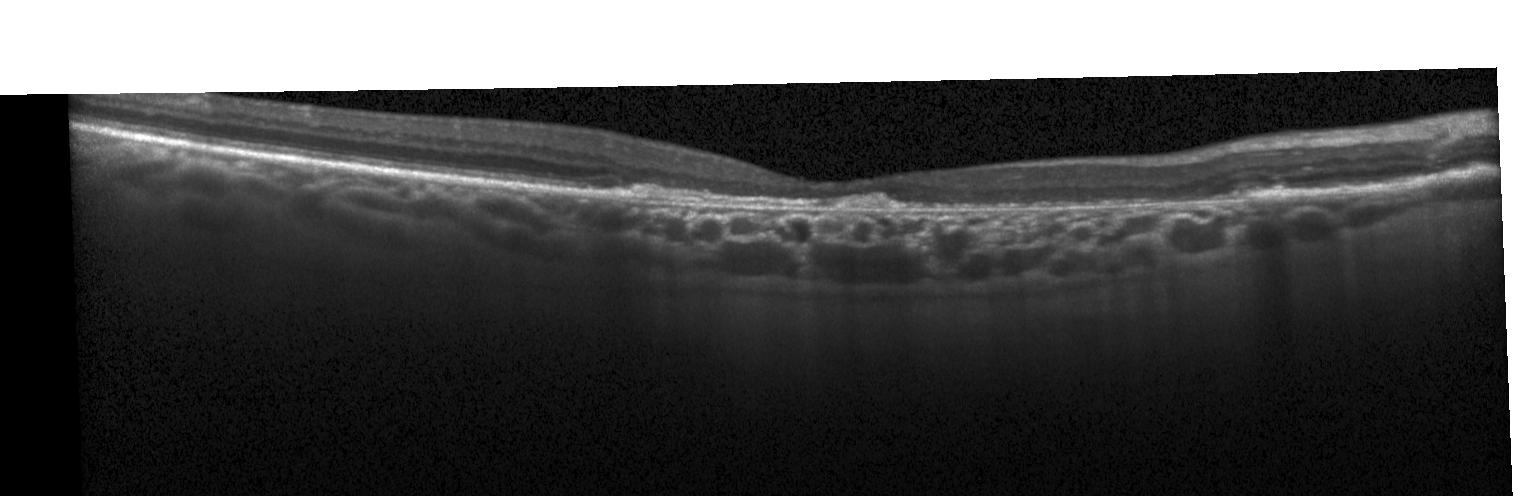 Spectral-domain OCT. OCT line scan. Finding: a choroidal neovascular membrane.